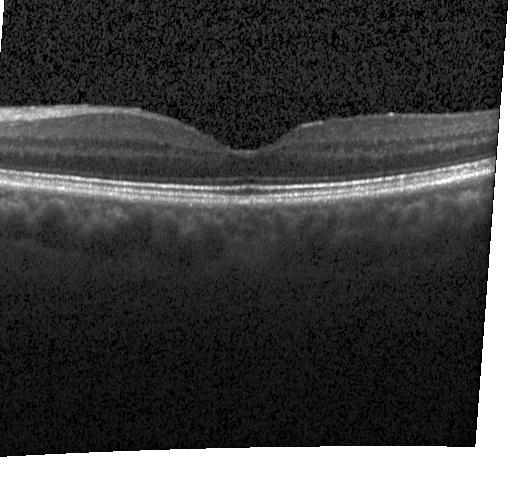

Impression: neither CNV, DME, nor drusen.